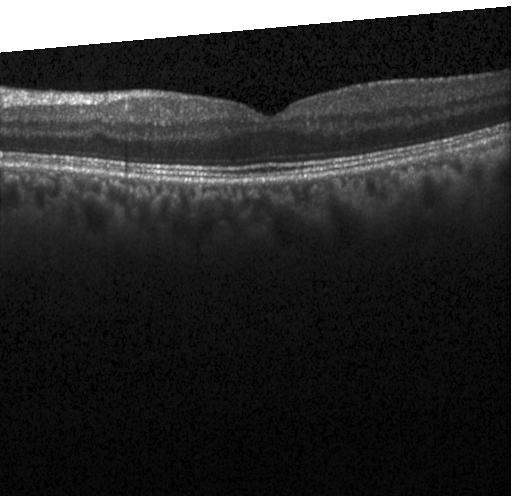

Optical coherence tomography scan — Dx: no choroidal neovascularization, diabetic macular edema, or drusen.